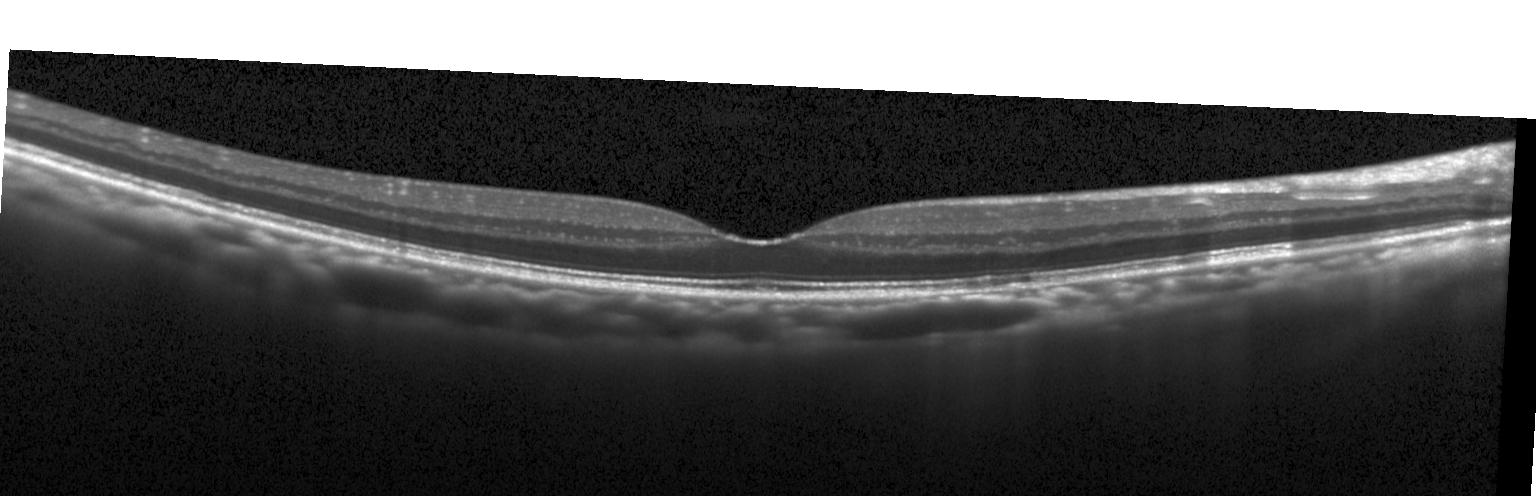

Retinal OCT B-scan · spectral-domain OCT · Heidelberg Spectralis · fovea-centered — Macular OCT: no choroidal neovascularization, no diabetic macular edema, and no drusen.